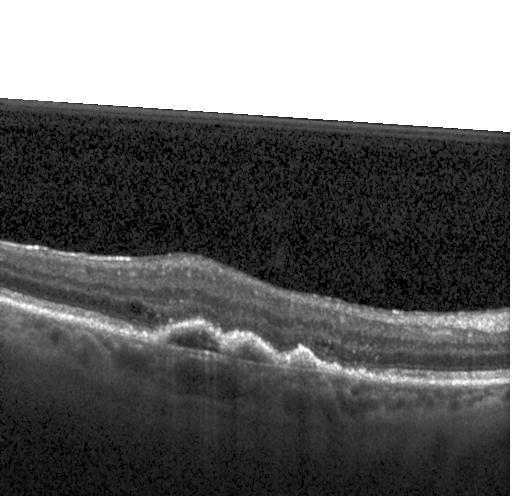

Assessment: a choroidal neovascular membrane.